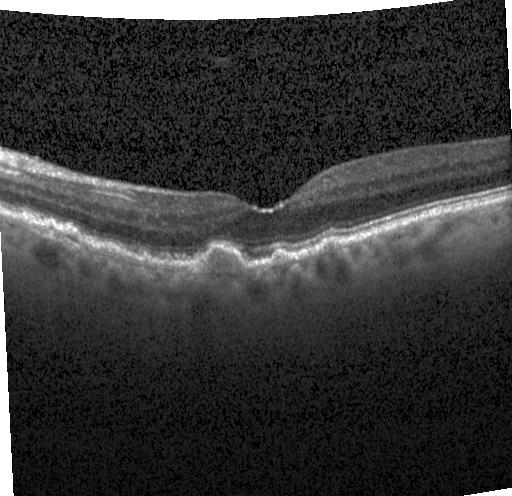 The scan shows drusen.